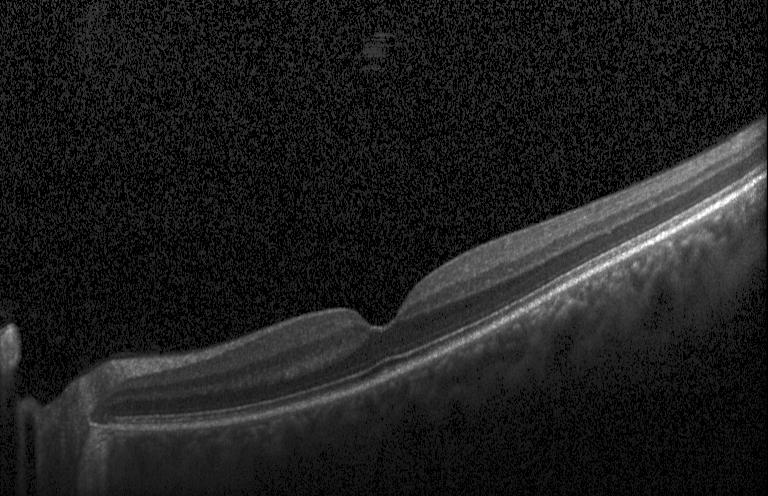 Impression: neither choroidal neovascularization, diabetic macular edema, nor drusen.